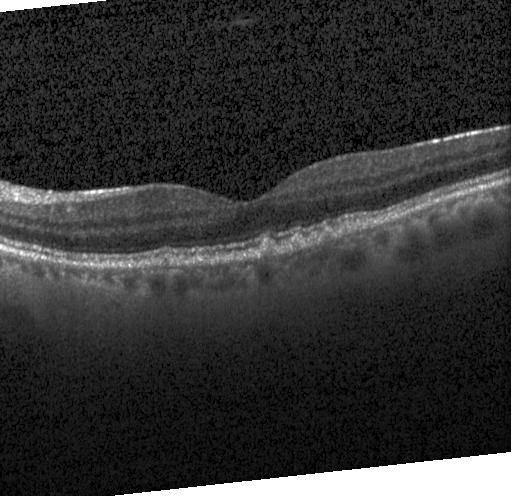 Horizontal scan through the fovea. Retinal OCT cross-section
This B-scan demonstrates sub-RPE drusenoid deposits.